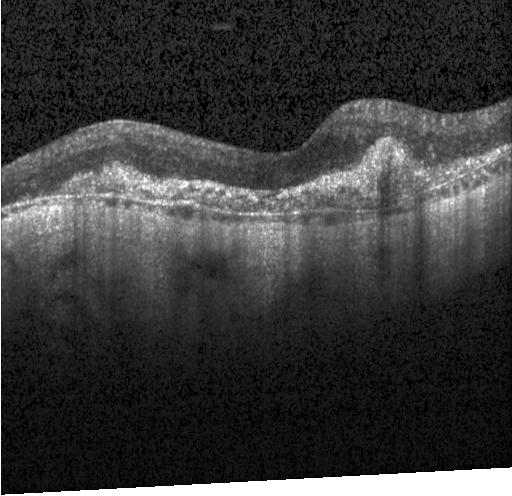
The scan shows CNV.